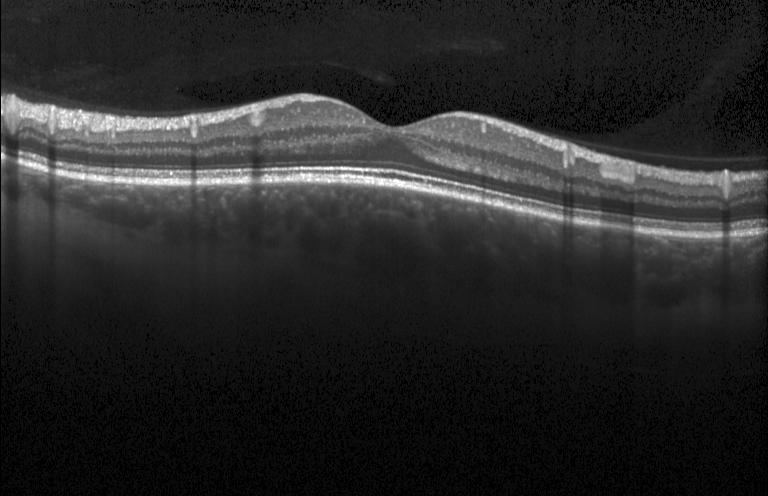
OCT B-scan — Finding: no evidence of choroidal neovascularization, diabetic macular edema, or drusen.